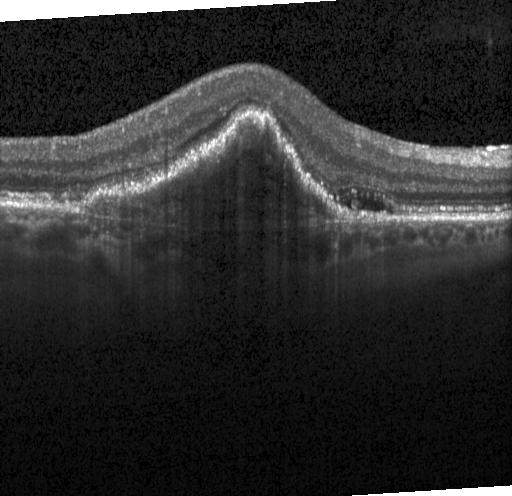 Centered on the fovea; acquired on a Heidelberg Spectralis; optical coherence tomography scan; SD-OCT.
Finding: a choroidal neovascular membrane.